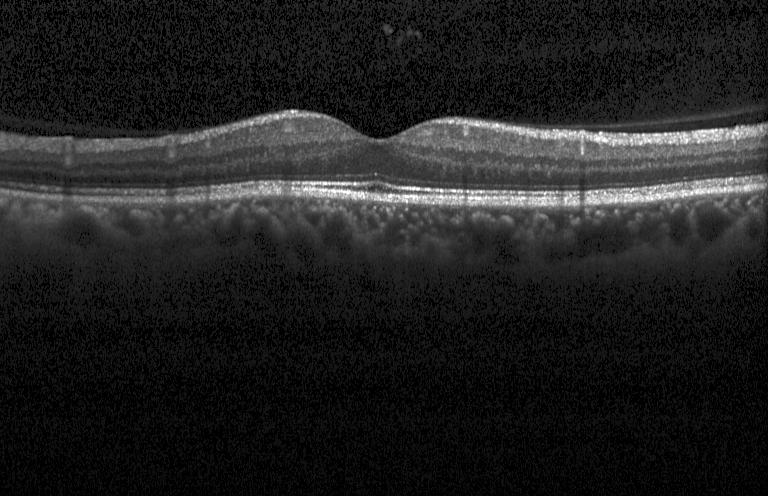 Macular OCT: no choroidal neovascularization, diabetic macular edema, or drusen.